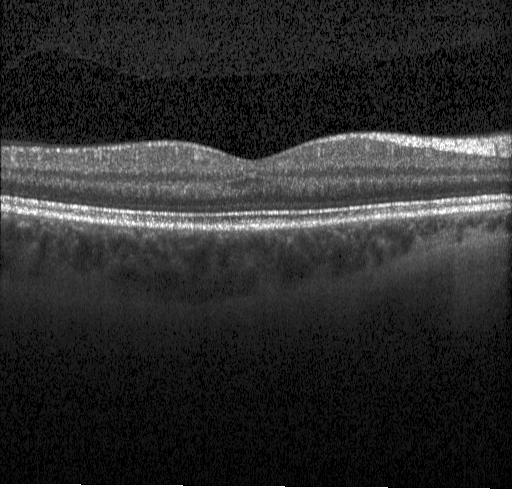 Retinal OCT cross-section, through the macula — Dx: no evidence of CNV, DME, or drusen.